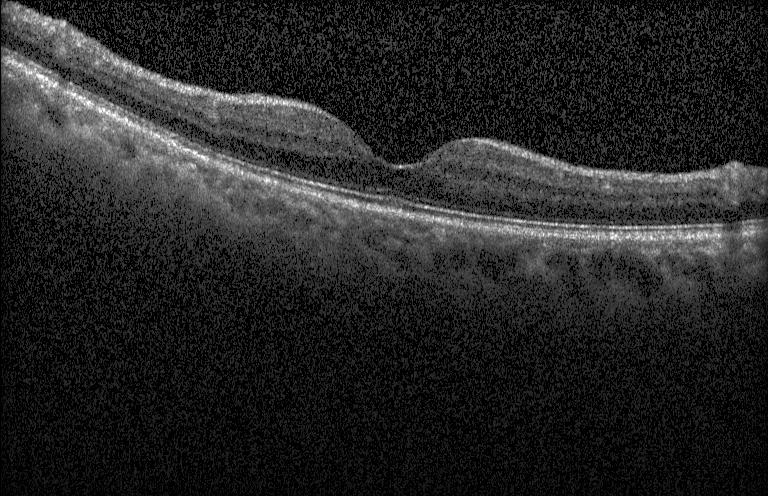
No CNV, no DME, and no drusen.